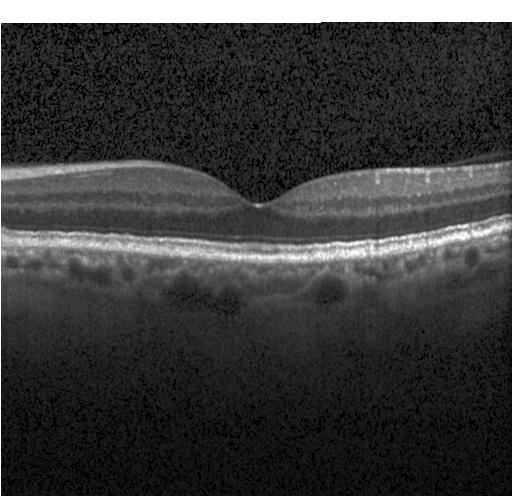 Horizontal scan through the fovea; retinal OCT B-scan — Finding: no evidence of CNV, DME, or drusen.